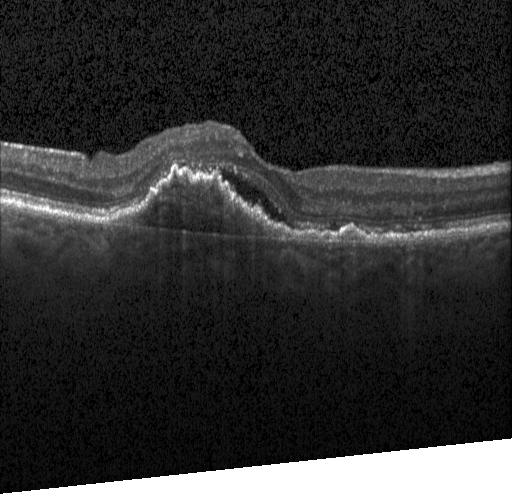
OCT finding: choroidal neovascularization (CNV).